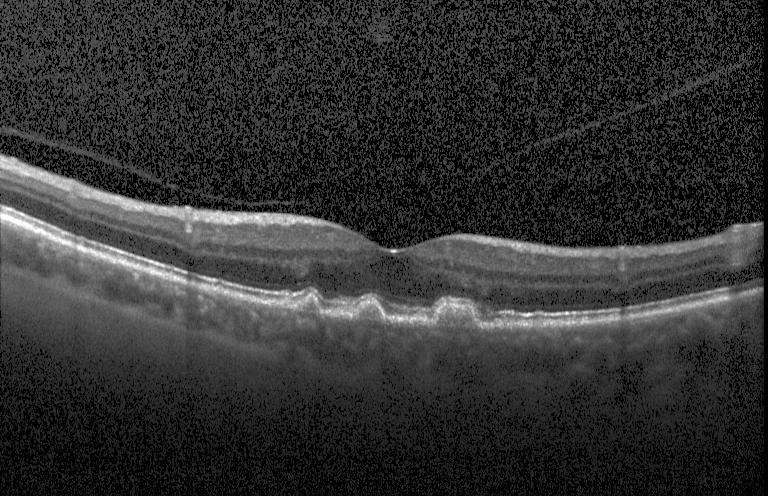

Heidelberg Spectralis. Retinal OCT cross-section. SD-OCT
Impression: drusen.